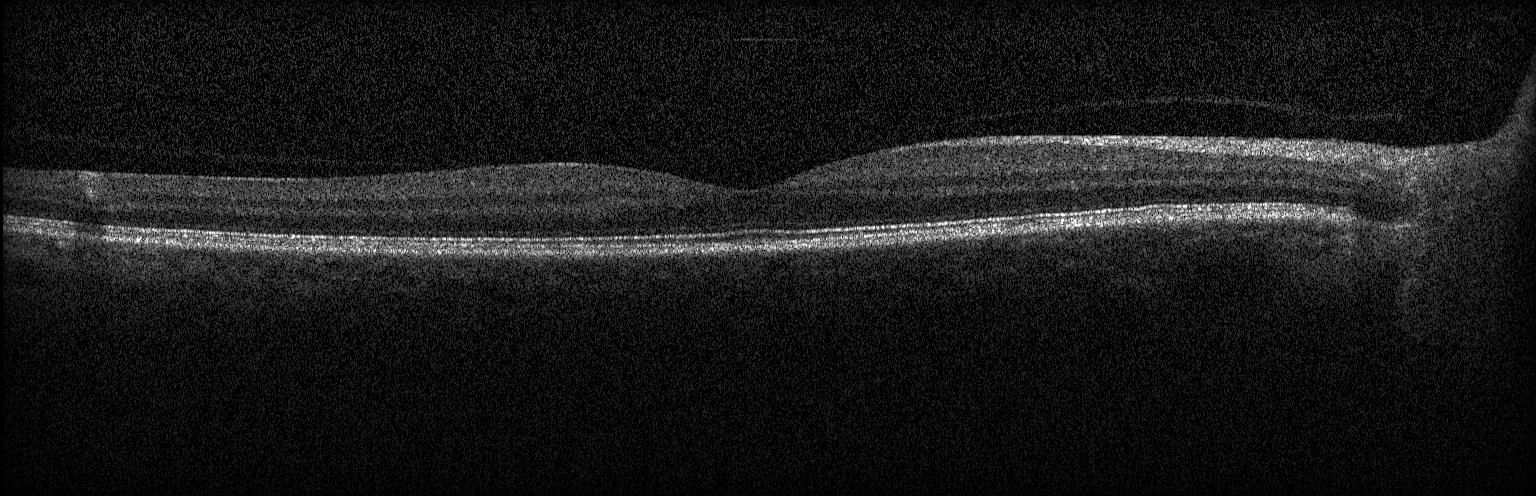
Optical coherence tomography scan.
Diagnosis: no choroidal neovascularization, diabetic macular edema, or drusen.